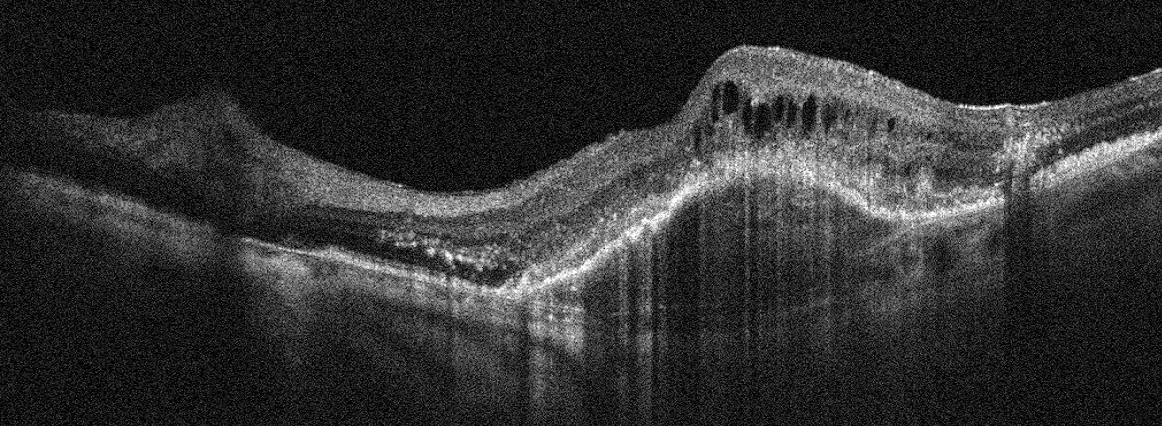
Left eye; optical coherence tomography scan.
The scan shows age-related macular degeneration.